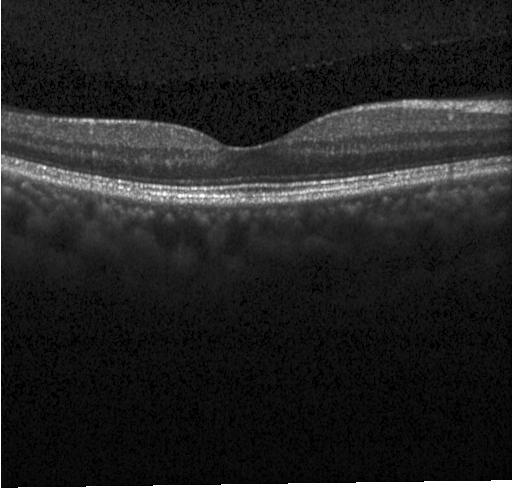
OCT line scan. This B-scan demonstrates neither choroidal neovascularization, diabetic macular edema, nor drusen.